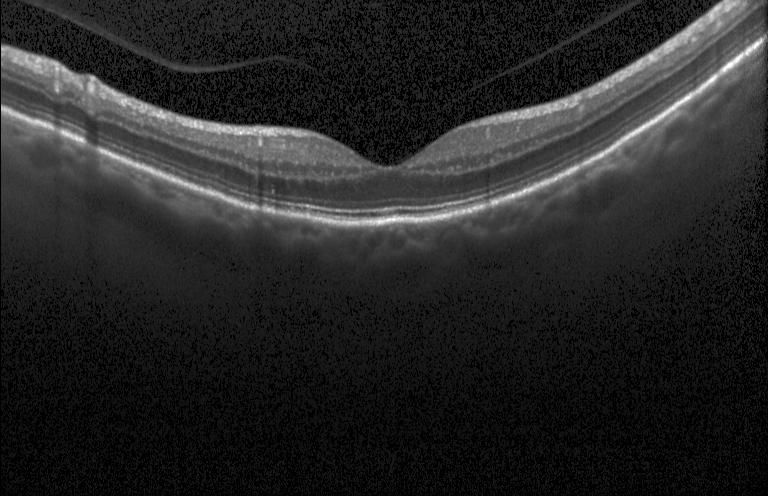

OCT line scan. Assessment: no evidence of choroidal neovascularization, diabetic macular edema, or drusen.